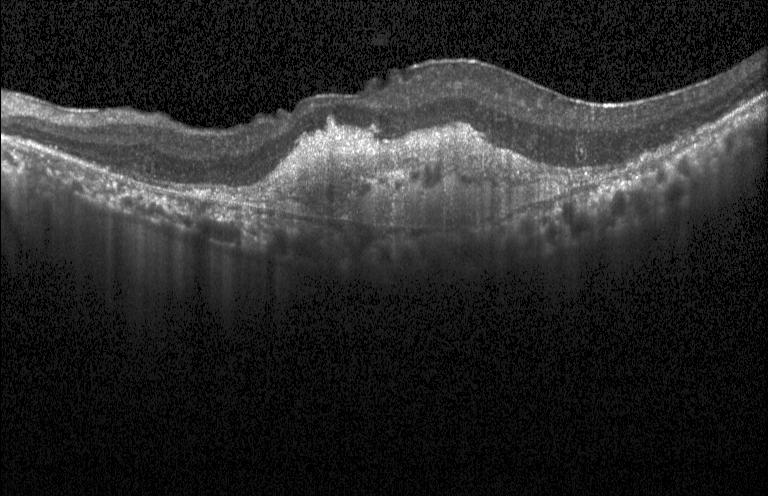 Diagnosis: a choroidal neovascular membrane.